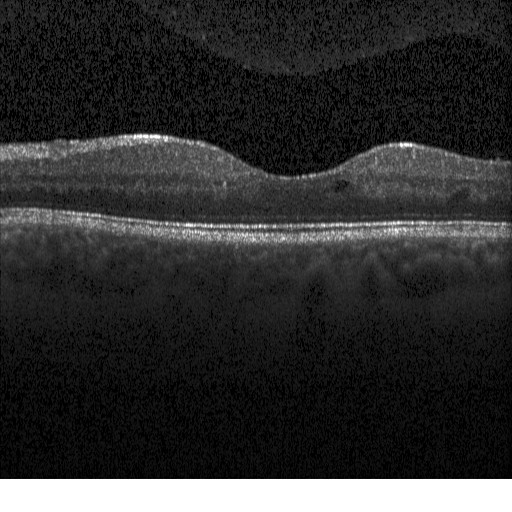
Macular OCT demonstrating diabetic macular edema (DME).